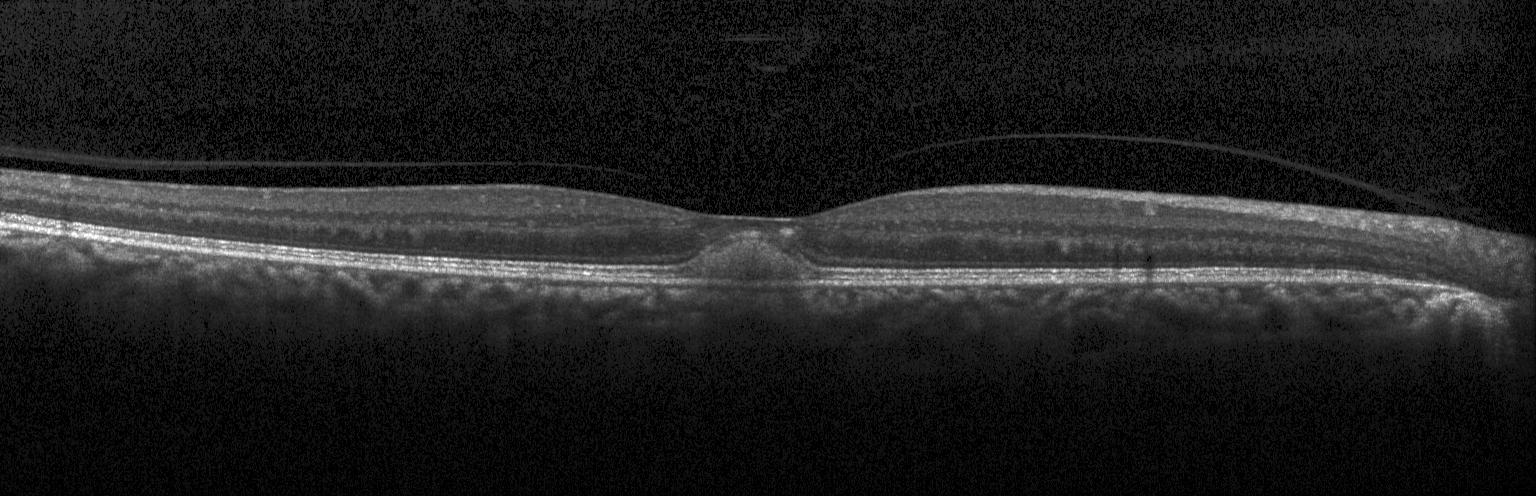

Spectral-domain optical coherence tomography · retinal OCT cross-section · Heidelberg Spectralis OCT system.
Impression: a choroidal neovascular membrane.